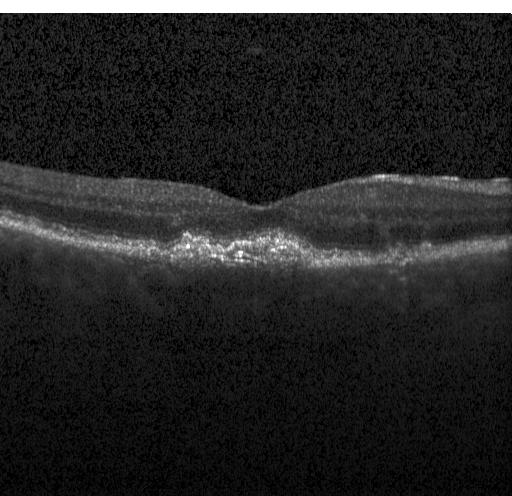
The scan shows choroidal neovascularization (CNV).